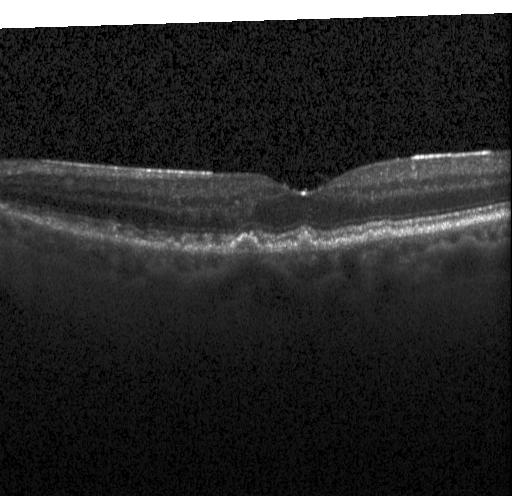

Finding: multiple drusen.